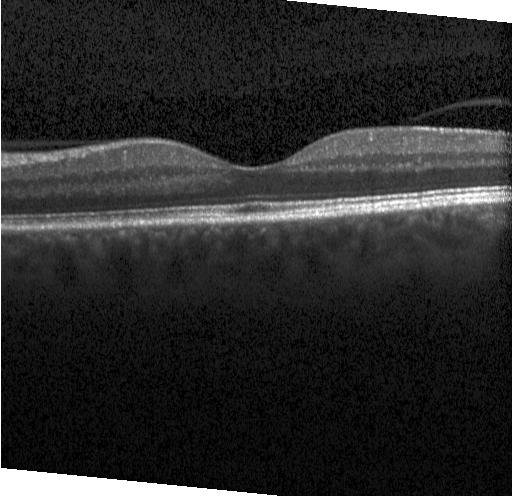

Fovea-centered. Spectral-domain OCT. OCT line scan
Finding: neither choroidal neovascularization, diabetic macular edema, nor drusen.